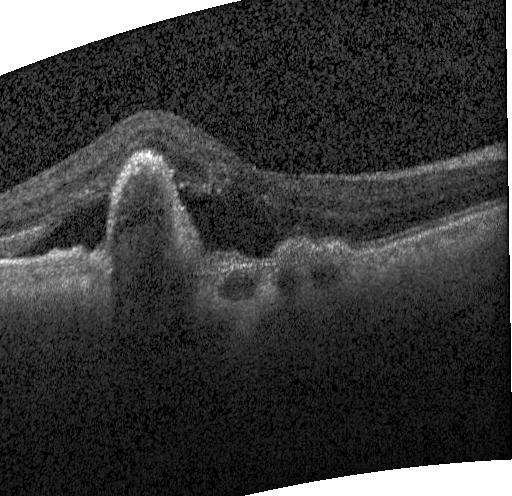 OCT B-scan.
Impression: a choroidal neovascular membrane.